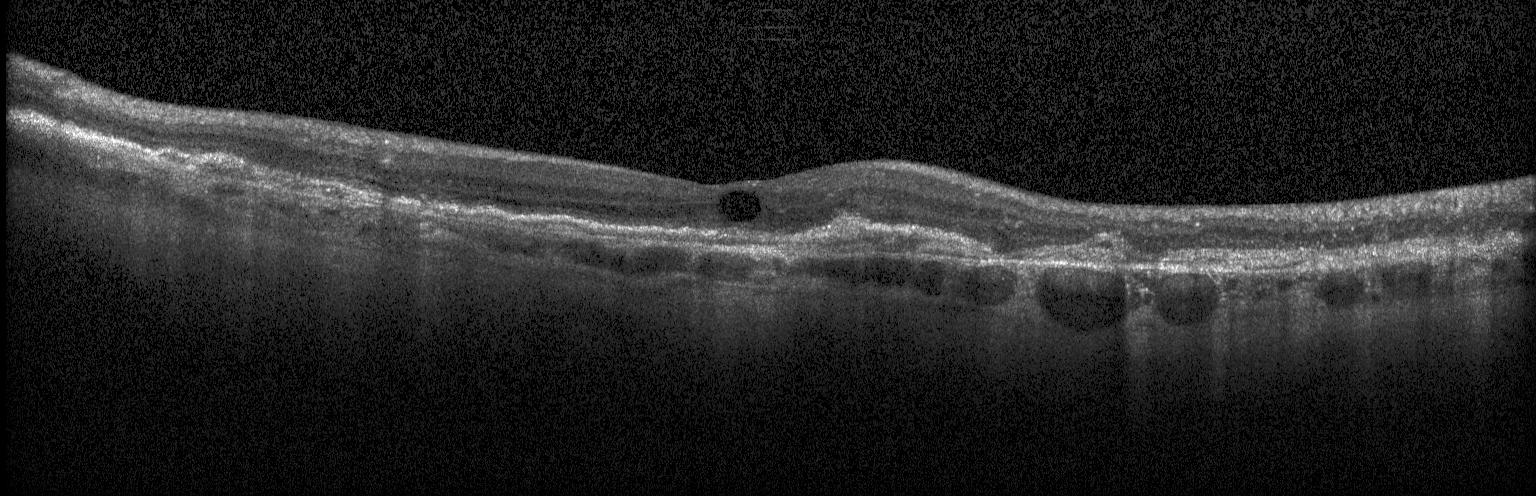 Heidelberg Spectralis OCT system; retinal OCT B-scan
This B-scan demonstrates a choroidal neovascular membrane.